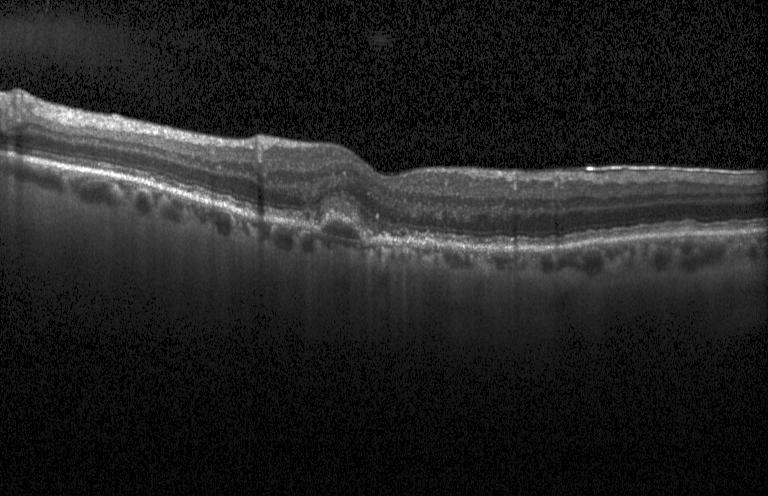

Horizontal scan through the fovea. Spectral-domain optical coherence tomography. Instrument: Heidelberg Spectralis. OCT B-scan
Finding: a choroidal neovascular membrane.